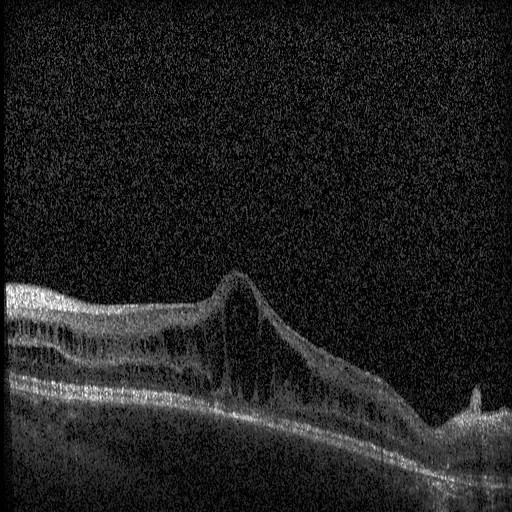 Retinal OCT B-scan.
This B-scan demonstrates diabetic macular edema.